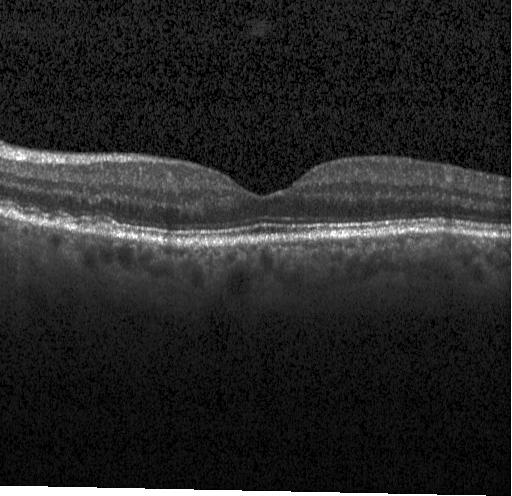

Retinal OCT cross-section · Heidelberg Spectralis · macular scan.
Impression: drusen.